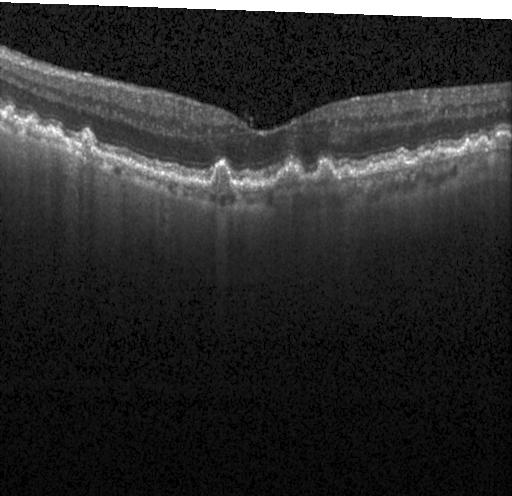
Spectral-domain OCT, Heidelberg Spectralis OCT system, OCT line scan
Impression: multiple drusen.